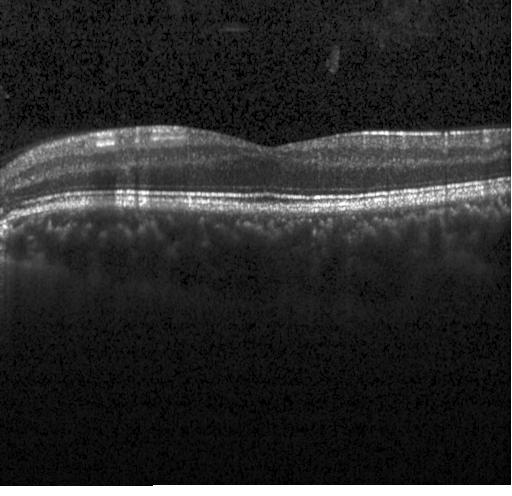

Spectral-domain OCT. Heidelberg Spectralis. Optical coherence tomography scan
The scan shows no choroidal neovascularization, diabetic macular edema, or drusen.